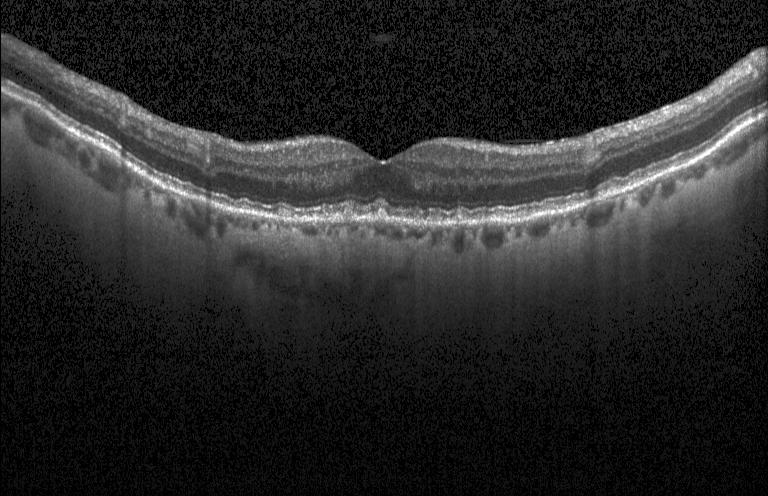 Retinal OCT cross-section · centered on the fovea · spectral-domain OCT — Drusen.